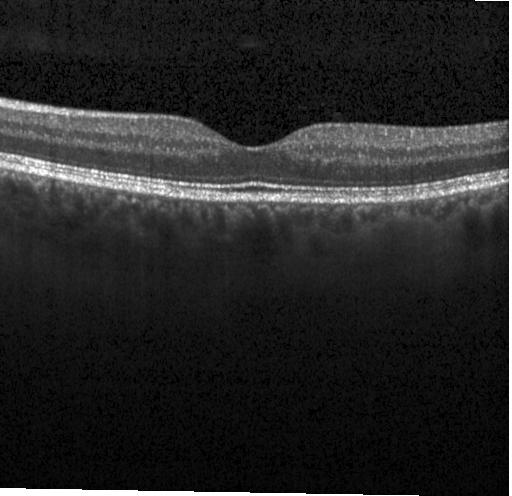
Retinal OCT B-scan. OCT finding: no choroidal neovascularization, diabetic macular edema, or drusen.